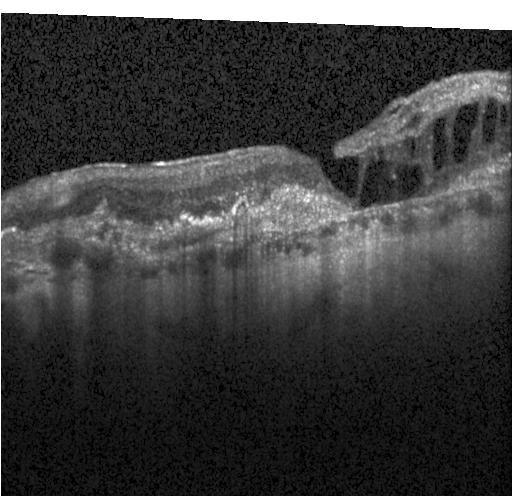
OCT line scan; instrument: Heidelberg Spectralis; fovea-centered; spectral-domain OCT. Diagnosis: a choroidal neovascular membrane.